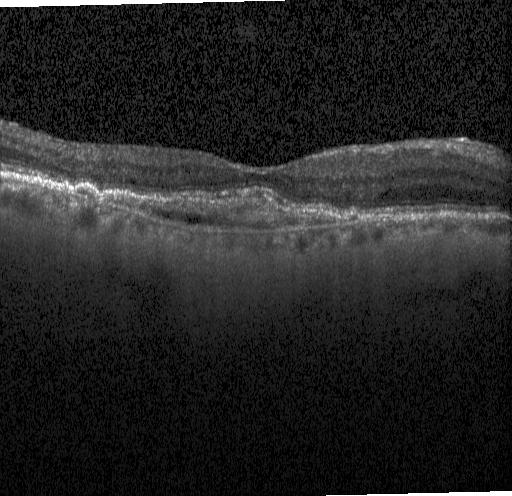 Macular scan. Spectral-domain OCT. OCT B-scan. Finding: a choroidal neovascular membrane.